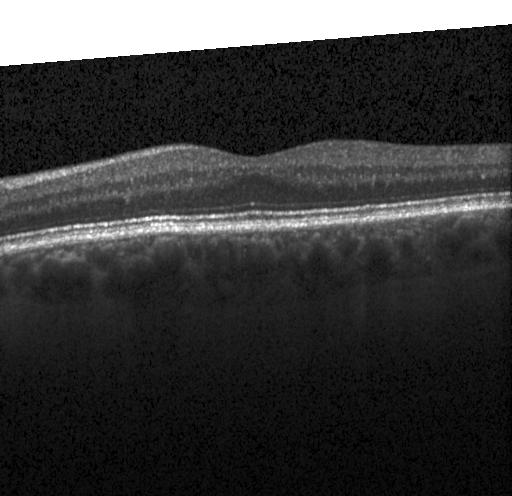

Optical coherence tomography B-scan, spectral-domain optical coherence tomography. Macular OCT: no choroidal neovascularization, no diabetic macular edema, and no drusen.